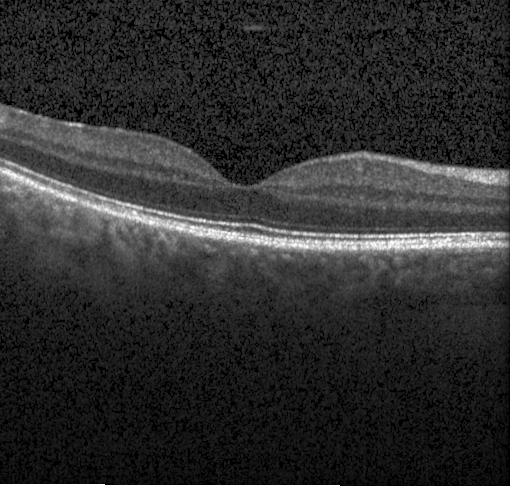
Assessment: neither CNV, DME, nor drusen.